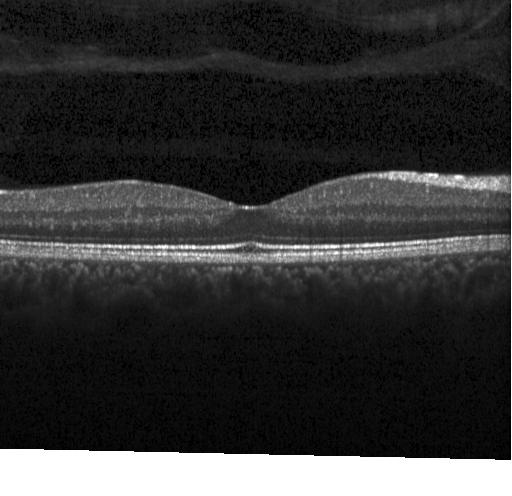
OCT finding: no evidence of CNV, DME, or drusen.